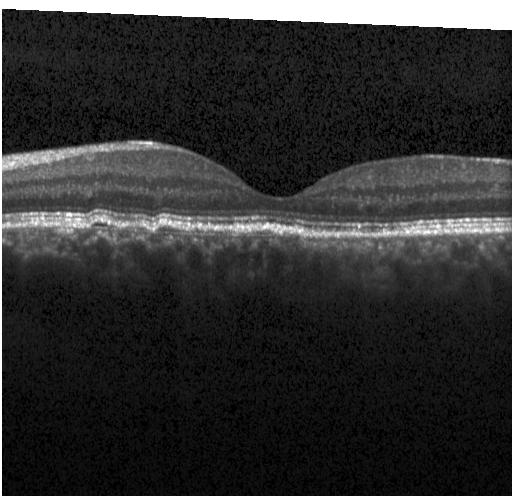
Spectral-domain OCT, Heidelberg Spectralis, horizontal scan through the fovea, optical coherence tomography B-scan.
Assessment: drusen.